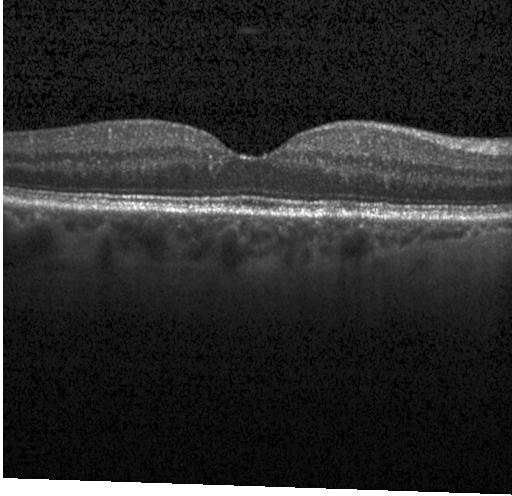 Through the macula · SD-OCT · optical coherence tomography B-scan · Heidelberg Spectralis OCT system.
Diagnosis: no choroidal neovascularization, no diabetic macular edema, and no drusen.